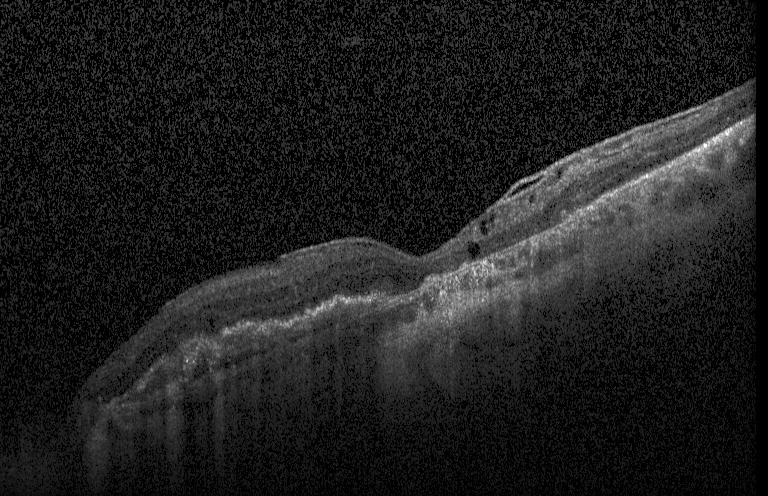

OCT B-scan, SD-OCT, horizontal scan through the fovea, Heidelberg Spectralis OCT system
A choroidal neovascular membrane.